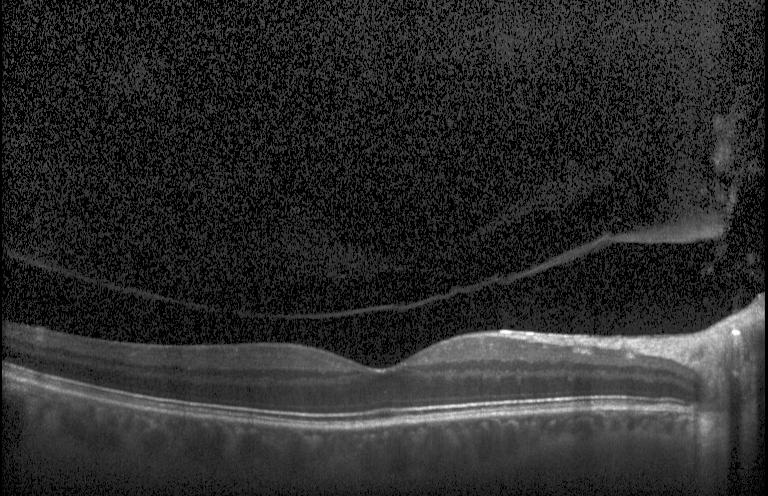 Instrument: Heidelberg Spectralis · macular scan · optical coherence tomography scan
This B-scan demonstrates neither choroidal neovascularization, diabetic macular edema, nor drusen.